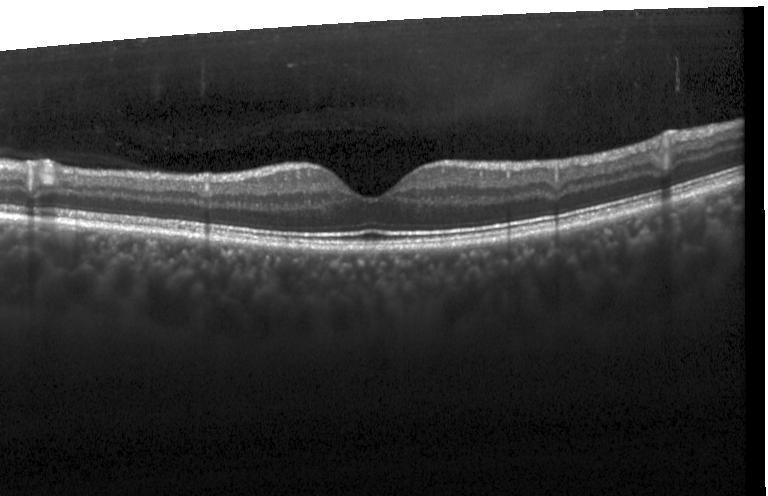 Retinal OCT cross-section showing no choroidal neovascularization, diabetic macular edema, or drusen.